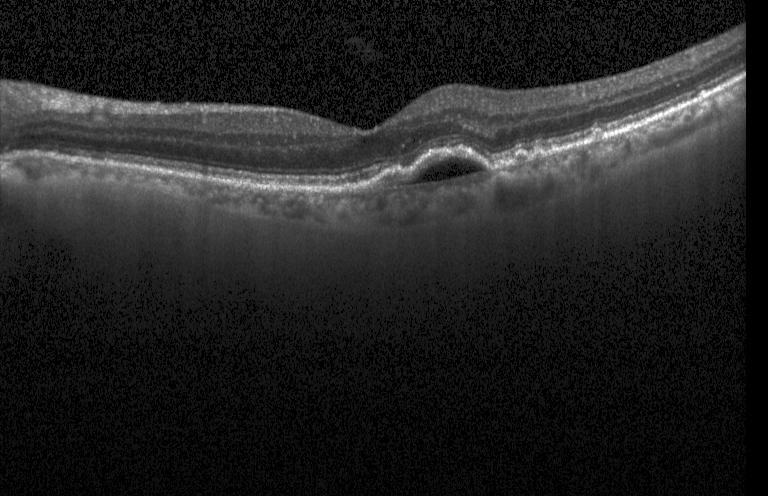
Retinal OCT B-scan — Finding: a choroidal neovascular membrane.